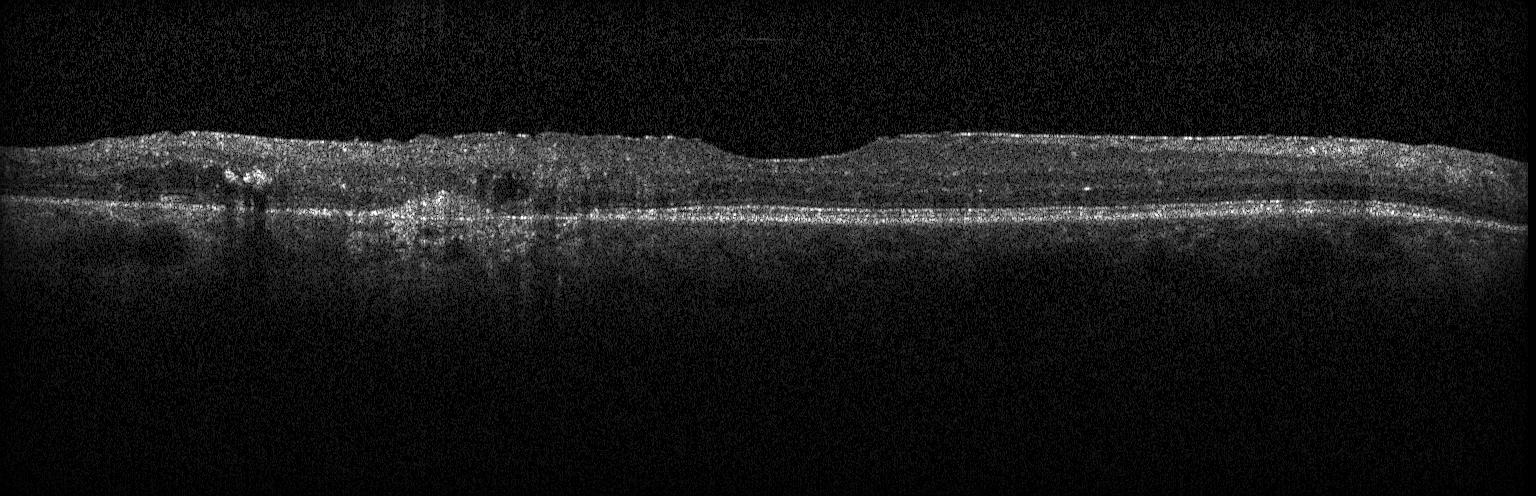 Retinal OCT cross-section showing a choroidal neovascular membrane.